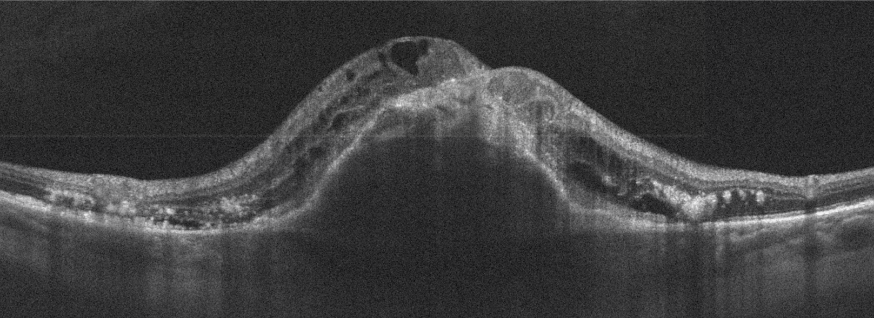
Optovue Avanti RTVue XR; macular scan; retinal OCT cross-section.
Diagnosis: age-related macular degeneration.